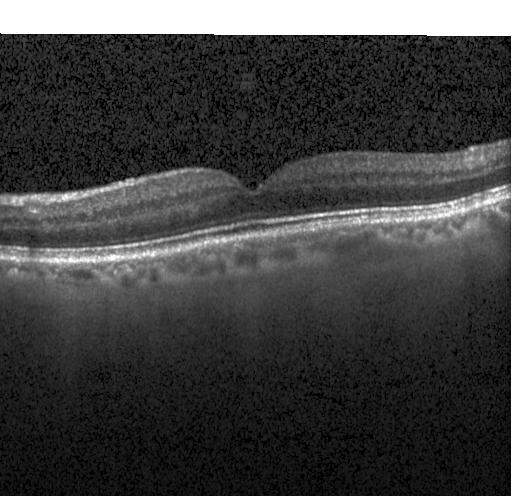
Optical coherence tomography scan. Instrument: Heidelberg Spectralis — Finding: no choroidal neovascularization, diabetic macular edema, or drusen.